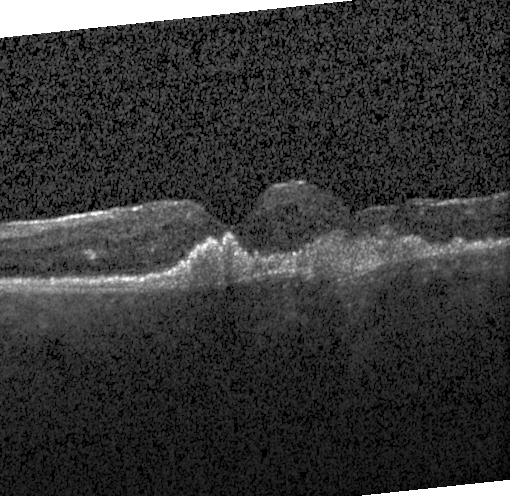

Retinal OCT B-scan; spectral-domain optical coherence tomography
Macular OCT: CNV.